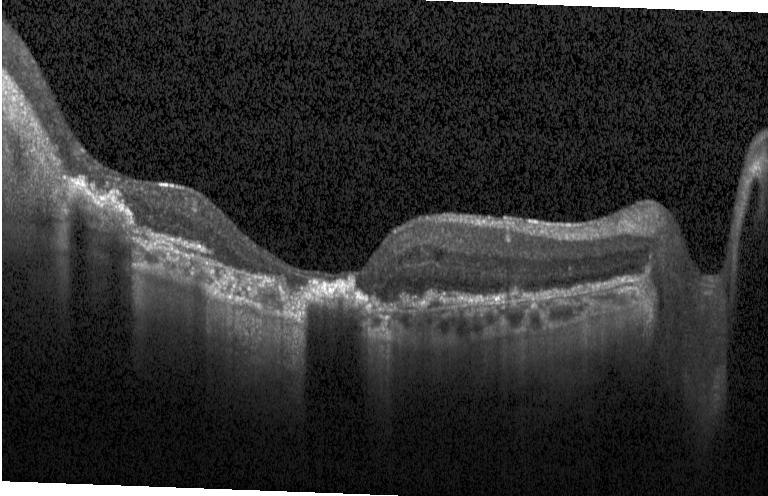 OCT line scan.
Impression: a choroidal neovascular membrane.